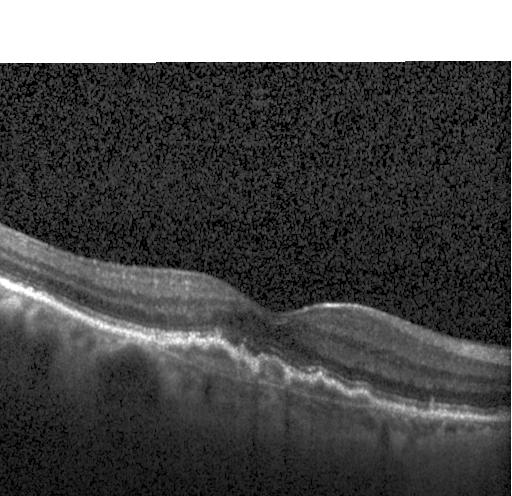
Impression: a choroidal neovascular membrane.